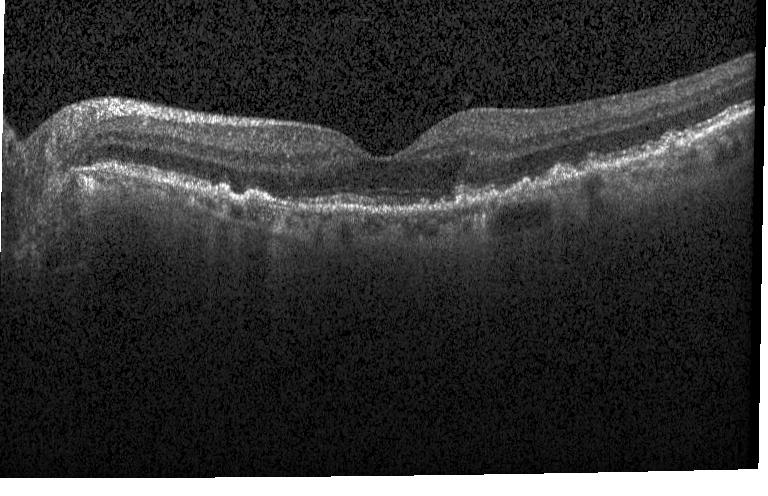

Diagnosis: drusen.